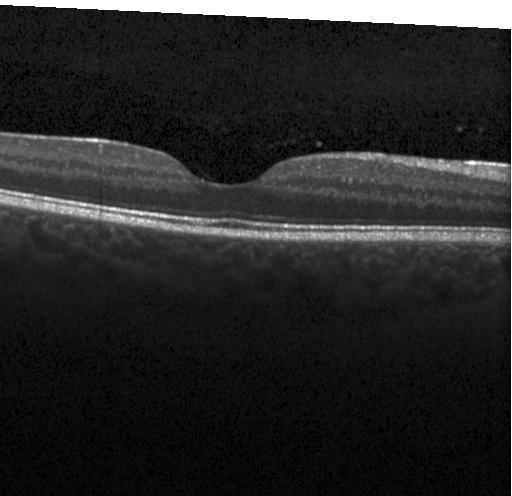 This B-scan demonstrates no choroidal neovascularization, diabetic macular edema, or drusen.